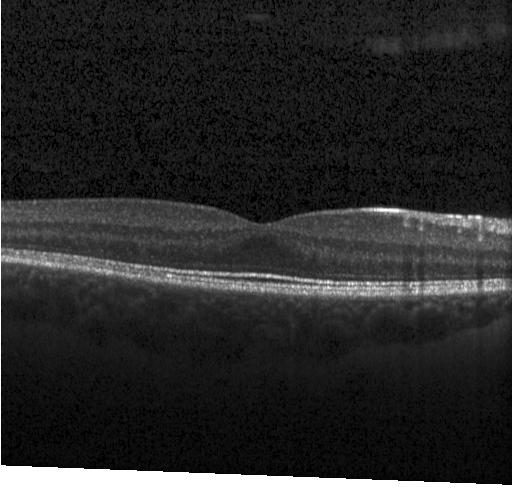

Diagnosis: neither choroidal neovascularization, diabetic macular edema, nor drusen.